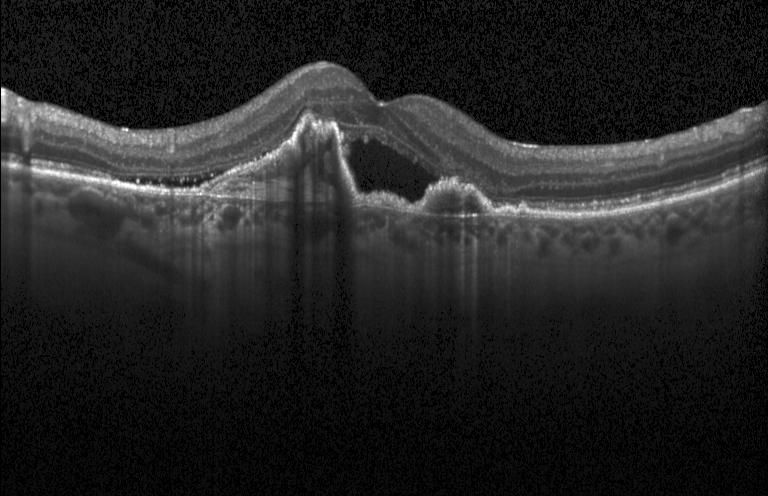
Macular OCT: a choroidal neovascular membrane.